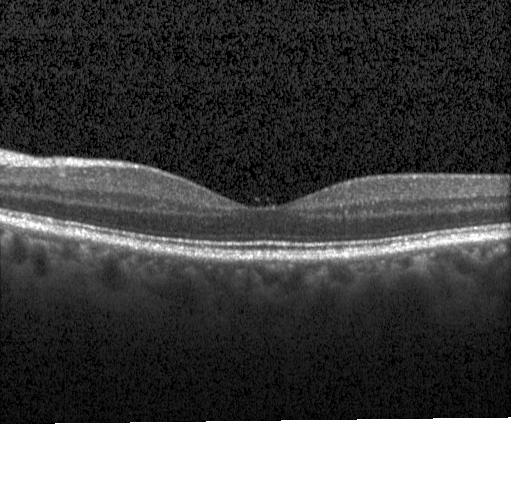
OCT scan showing neither CNV, DME, nor drusen.